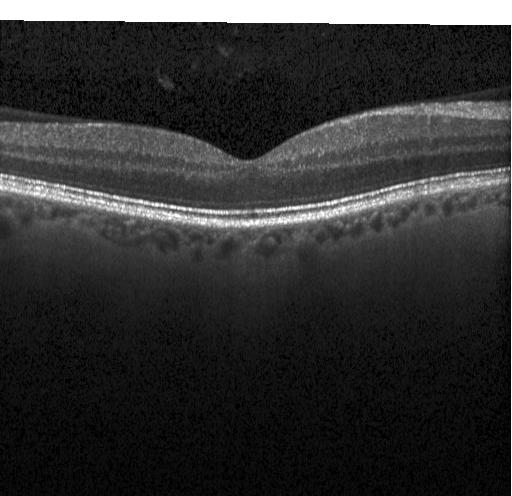

Optical coherence tomography scan. Horizontal scan through the fovea. Neither choroidal neovascularization, diabetic macular edema, nor drusen.